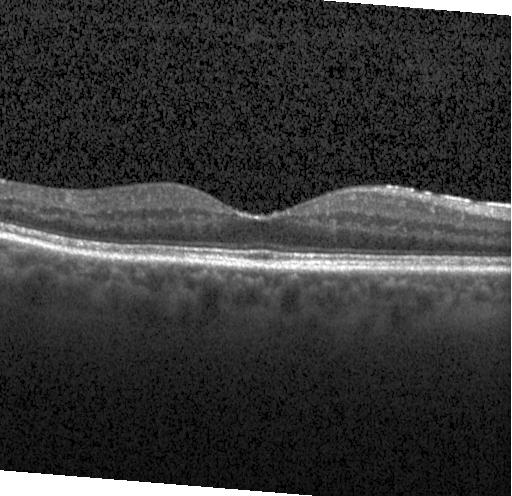
OCT B-scan. Assessment: no choroidal neovascularization, no diabetic macular edema, and no drusen.